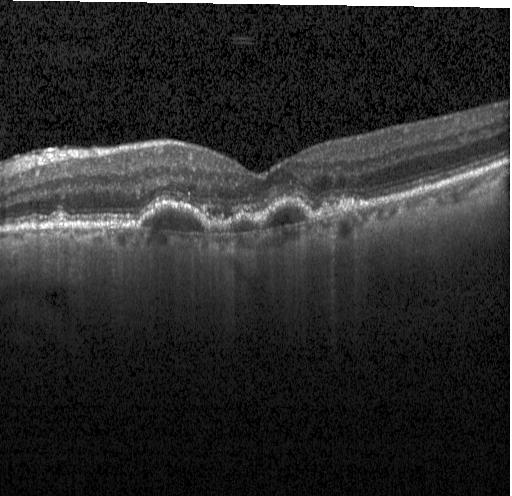 Acquired on a Heidelberg Spectralis · through the macula · OCT B-scan — Dx: a choroidal neovascular membrane.